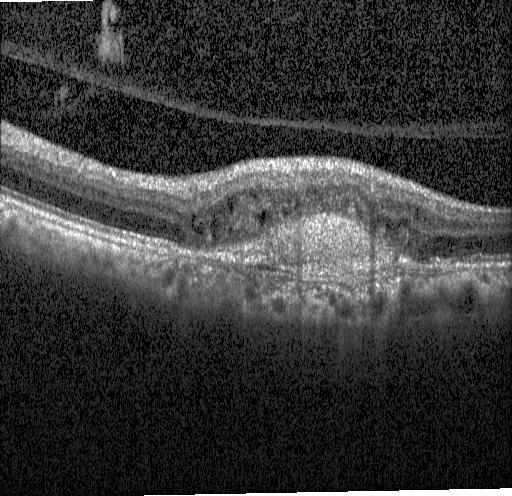 Spectral-domain OCT, Heidelberg Spectralis OCT system, through the macula, optical coherence tomography scan — Impression: a choroidal neovascular membrane.